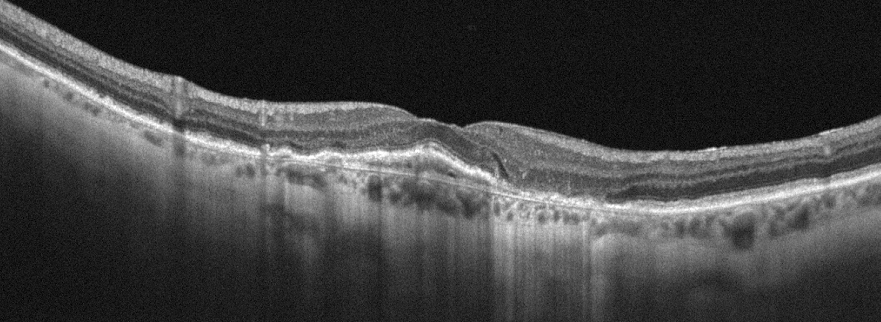

Macular scan; retinal OCT cross-section.
Finding: age-related macular degeneration.